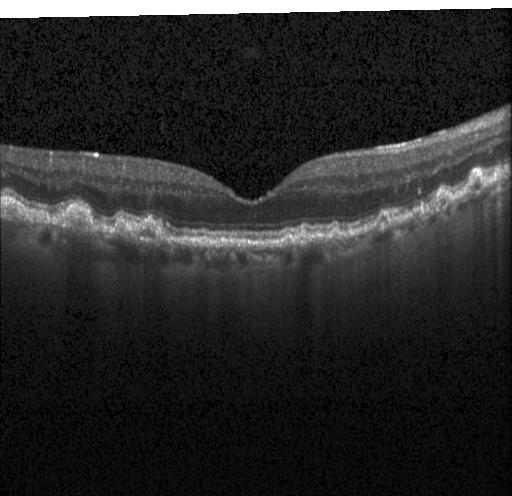

Horizontal scan through the fovea, retinal OCT B-scan. Sub-RPE drusenoid deposits.